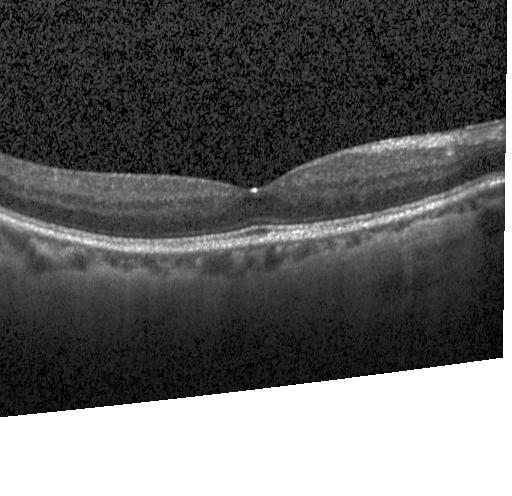

Dx: no CNV, DME, or drusen.